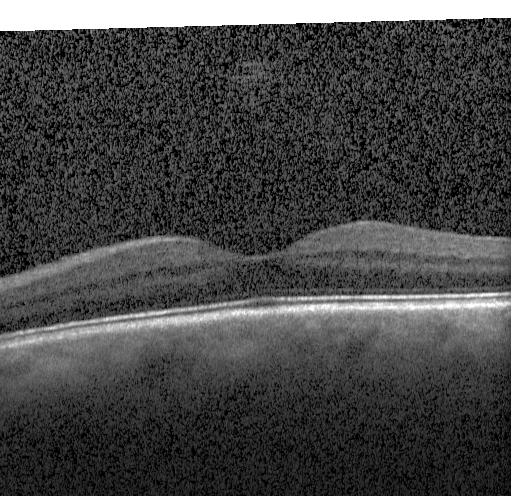 OCT line scan.
This B-scan demonstrates neither CNV, DME, nor drusen.